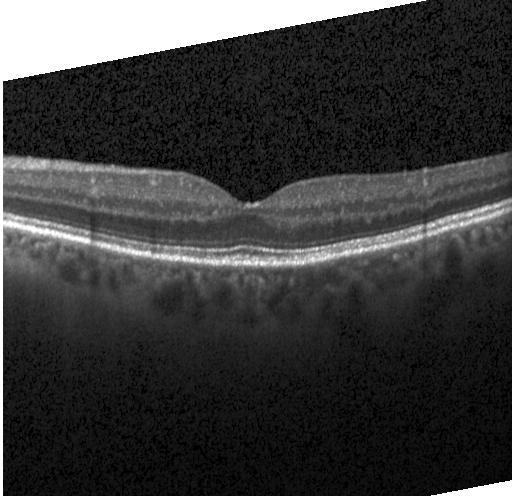
Optical coherence tomography scan, acquired on a Heidelberg Spectralis, centered on the fovea, spectral-domain optical coherence tomography. This B-scan demonstrates no evidence of CNV, DME, or drusen.